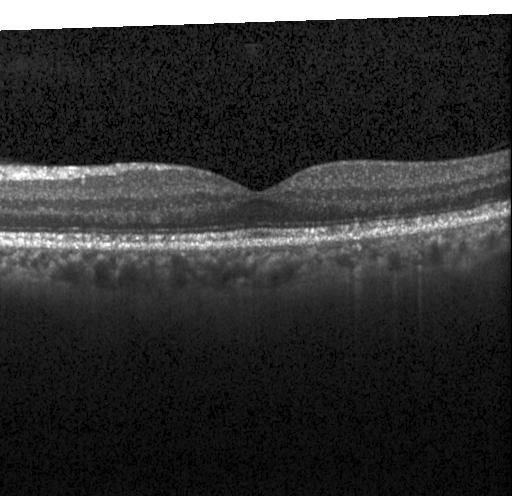

Spectral-domain optical coherence tomography, Heidelberg Spectralis, optical coherence tomography B-scan
Impression: no choroidal neovascularization, diabetic macular edema, or drusen.